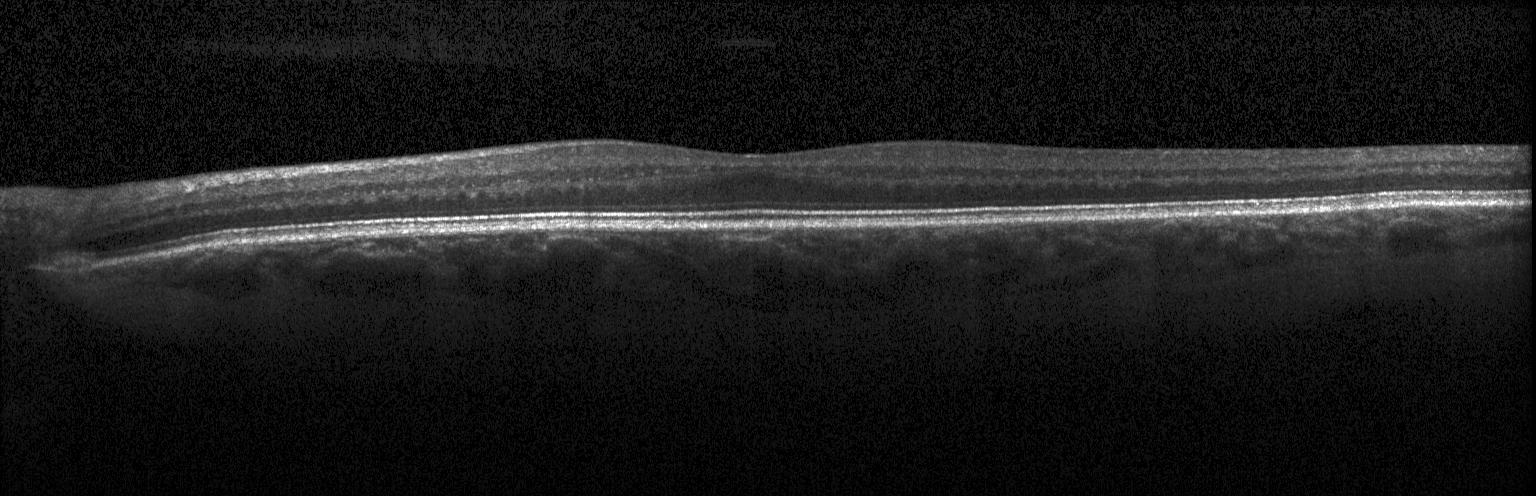
This B-scan demonstrates no evidence of choroidal neovascularization, diabetic macular edema, or drusen.